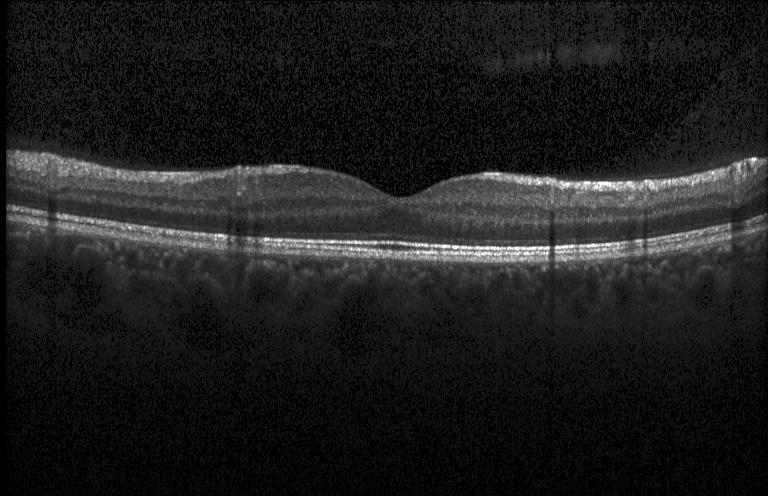

Macular OCT: neither choroidal neovascularization, diabetic macular edema, nor drusen.